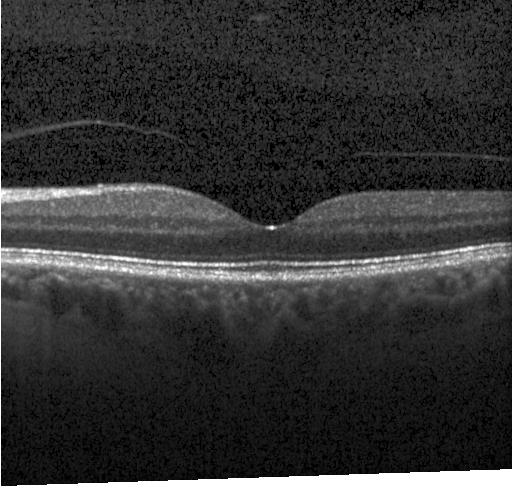
Spectral-domain optical coherence tomography. Retinal OCT cross-section. Dx: neither choroidal neovascularization, diabetic macular edema, nor drusen.